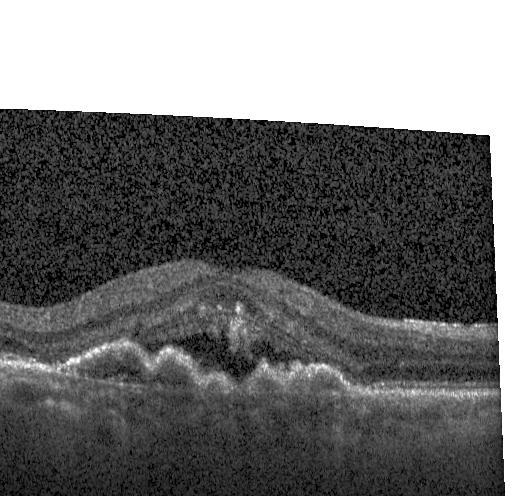
OCT B-scan
The scan shows CNV.